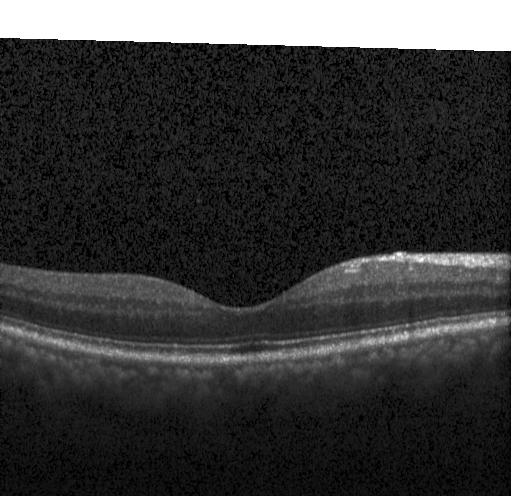

OCT line scan. Dx: no evidence of choroidal neovascularization, diabetic macular edema, or drusen.